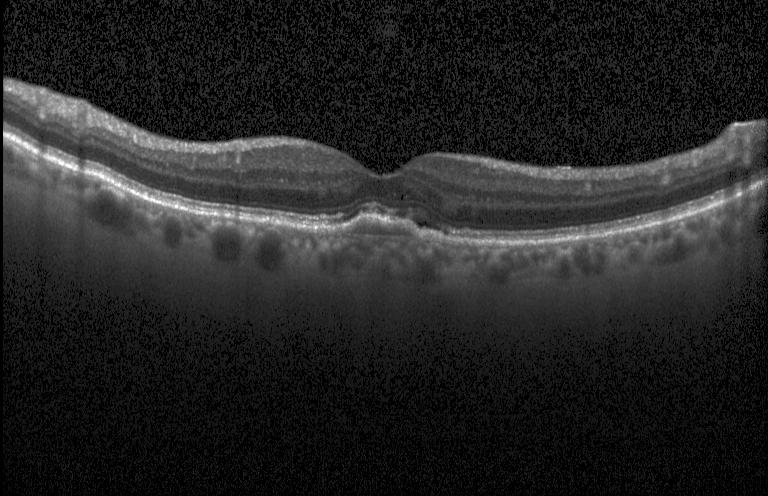 SD-OCT, retinal OCT cross-section
OCT finding: choroidal neovascularization.